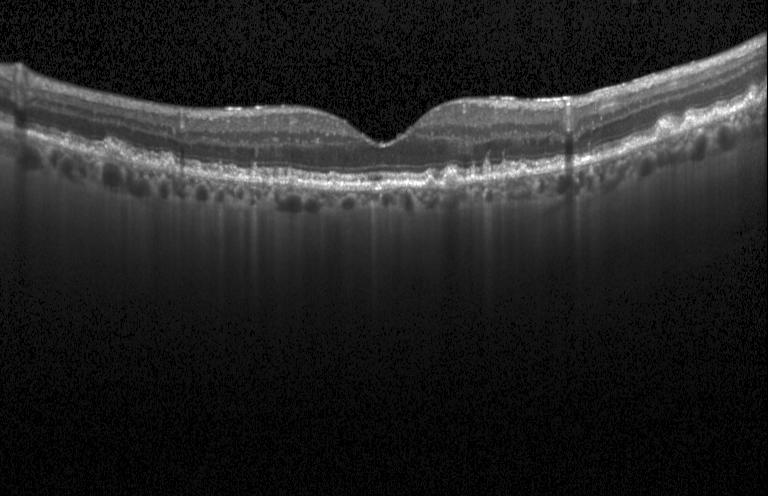
Finding: multiple drusen.